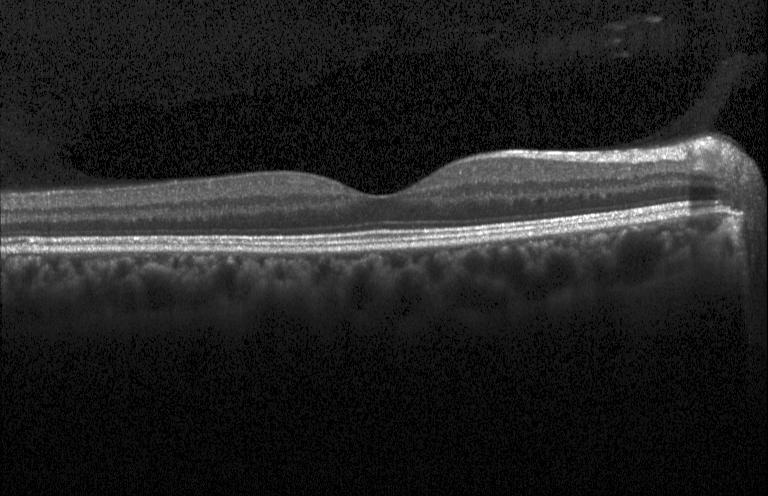
OCT scan showing no choroidal neovascularization, diabetic macular edema, or drusen.